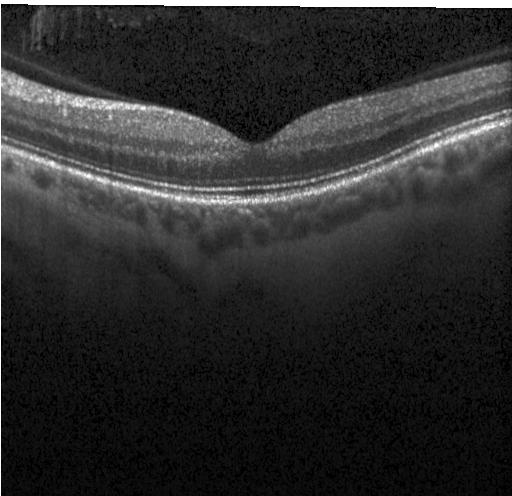
Finding: no choroidal neovascularization, diabetic macular edema, or drusen.